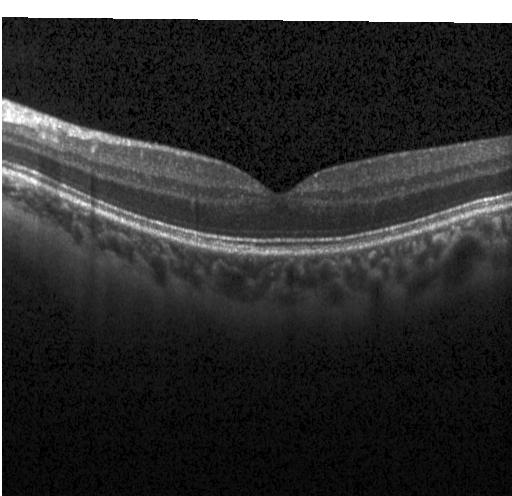 This B-scan demonstrates no evidence of CNV, DME, or drusen.